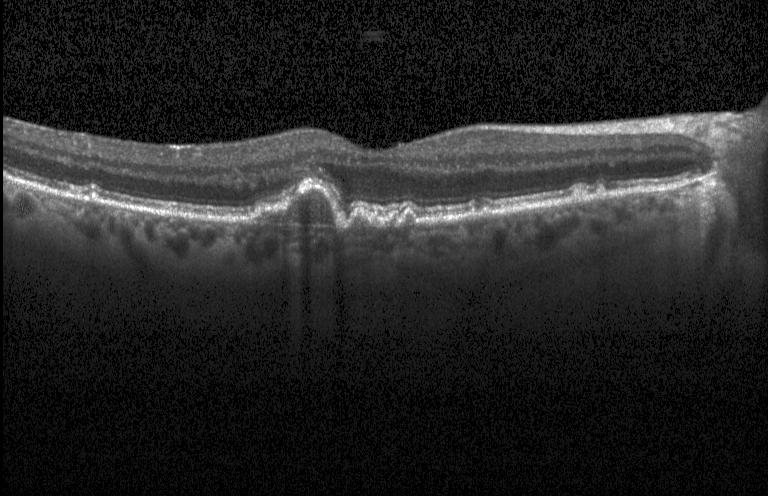

Heidelberg Spectralis OCT system · optical coherence tomography B-scan · horizontal scan through the fovea. Impression: multiple drusen.